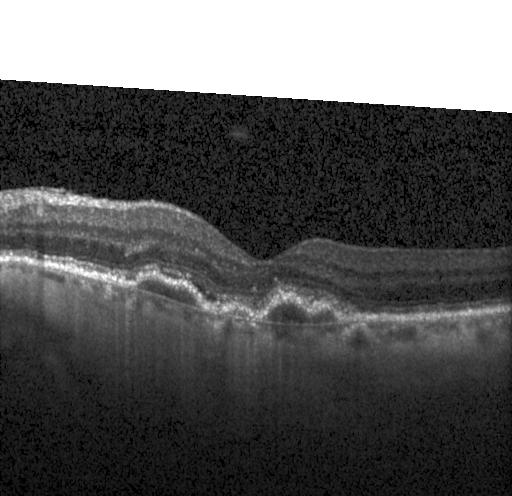

Heidelberg Spectralis OCT system. SD-OCT. OCT line scan. Through the macula.
Impression: a choroidal neovascular membrane.